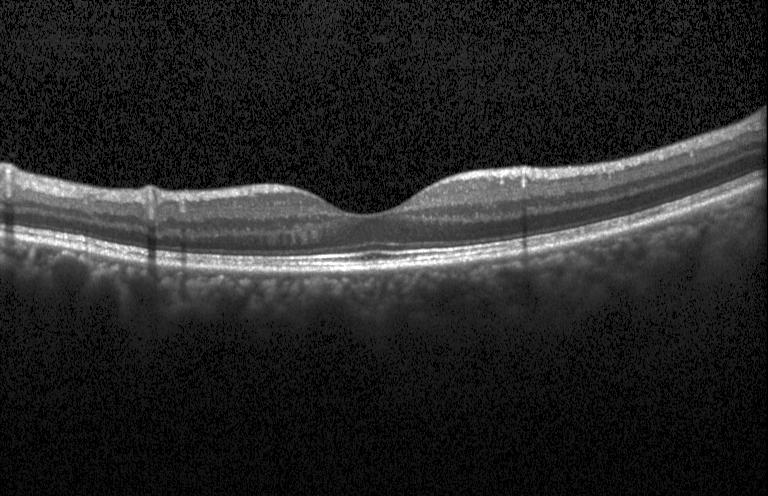

Retinal OCT B-scan; spectral-domain optical coherence tomography. Diagnosis: neither CNV, DME, nor drusen.